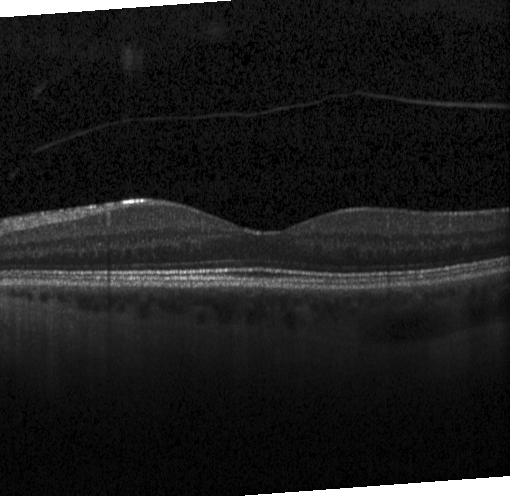
OCT B-scan.
Macular OCT: no evidence of choroidal neovascularization, diabetic macular edema, or drusen.